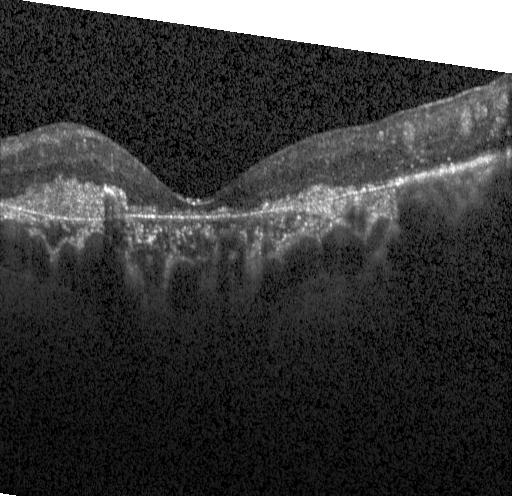

Optical coherence tomography B-scan.
Impression: a choroidal neovascular membrane.